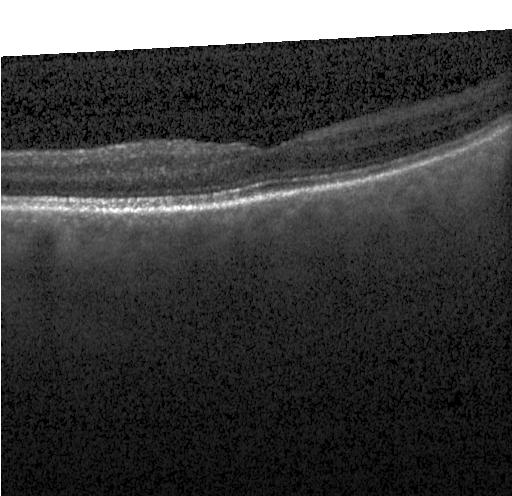 OCT finding: no CNV, DME, or drusen.